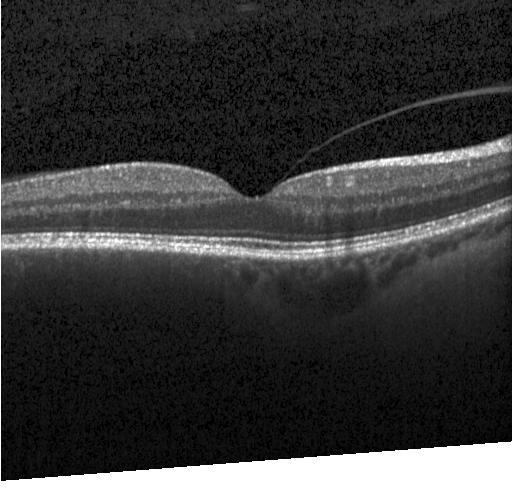 Spectral-domain OCT, macular scan, Heidelberg Spectralis, retinal OCT cross-section.
Impression: no choroidal neovascularization, no diabetic macular edema, and no drusen.